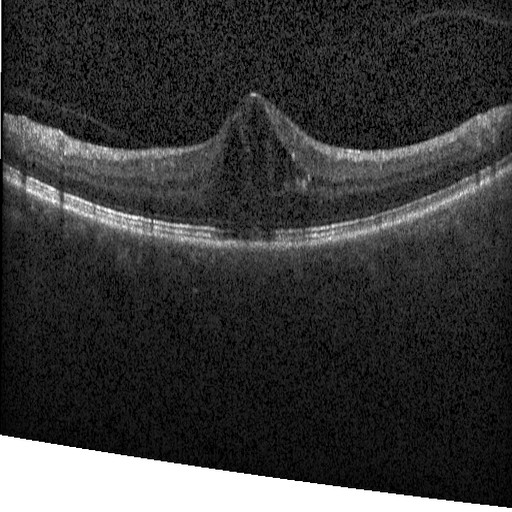

Centered on the fovea. OCT line scan. Heidelberg Spectralis. Spectral-domain OCT.
Impression: diabetic macular edema (DME).